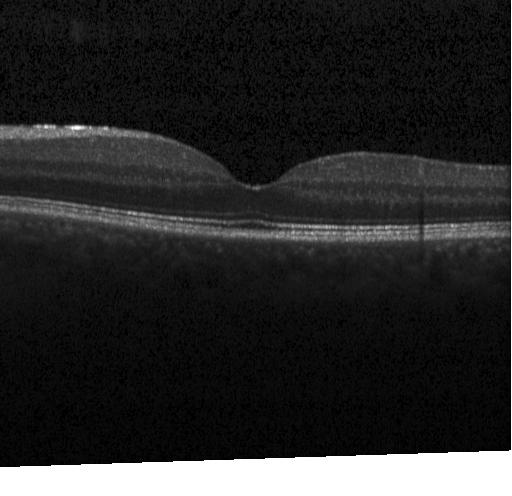

Macular OCT: no evidence of choroidal neovascularization, diabetic macular edema, or drusen.